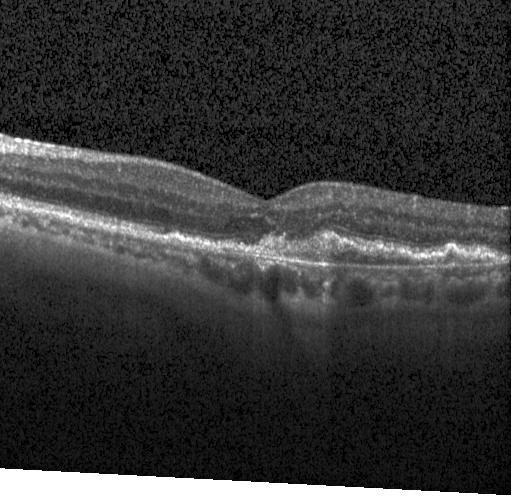
OCT B-scan.
The scan shows a choroidal neovascular membrane.